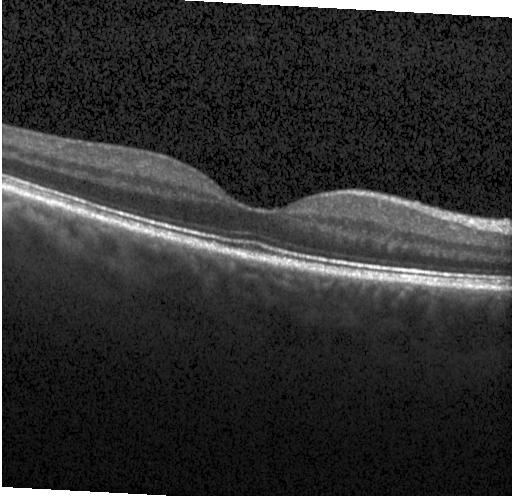
Assessment: no evidence of CNV, DME, or drusen.